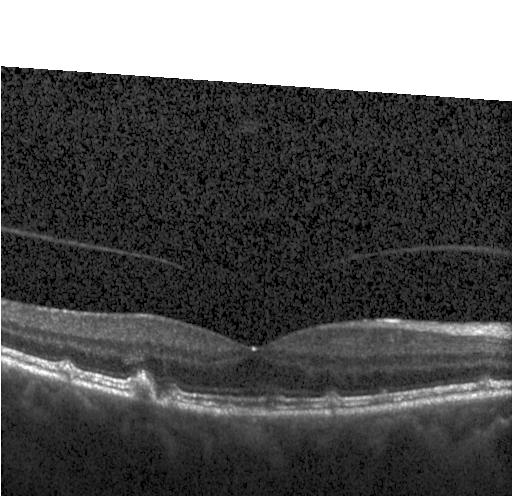 Retinal OCT cross-section
Macular OCT: multiple drusen.